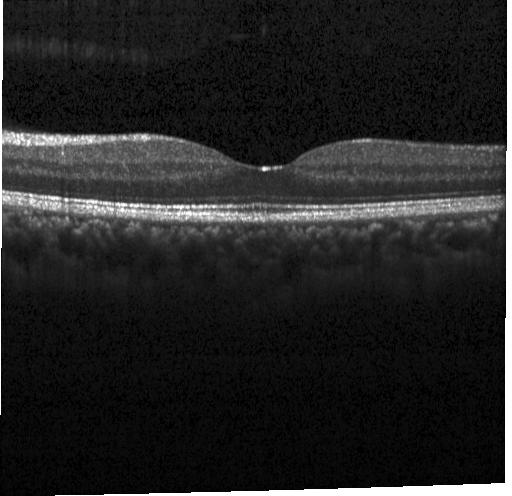
Retinal OCT cross-section showing no evidence of CNV, DME, or drusen.